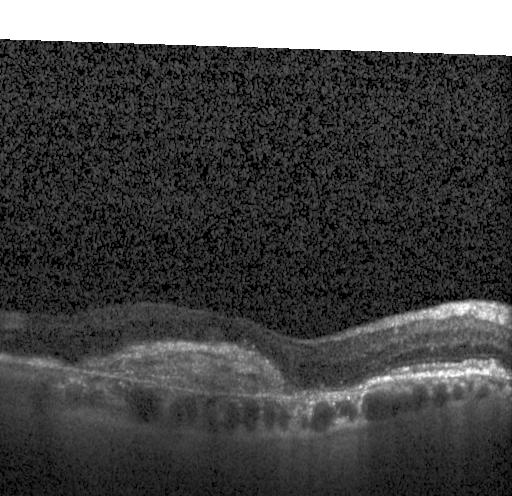

OCT line scan.
Macular OCT: choroidal neovascularization (CNV).